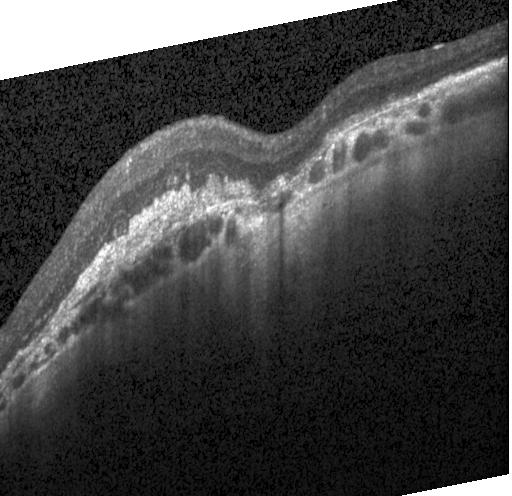

Dx: a choroidal neovascular membrane.